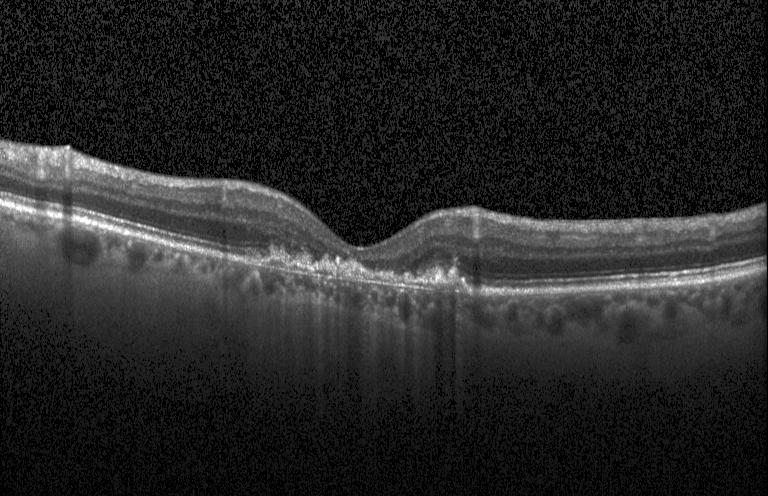

Optical coherence tomography scan. Impression: a choroidal neovascular membrane.